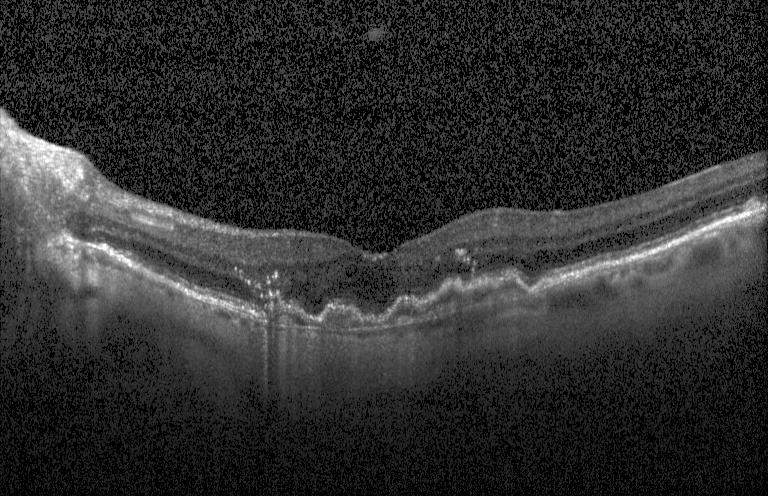 Macular OCT demonstrating CNV.